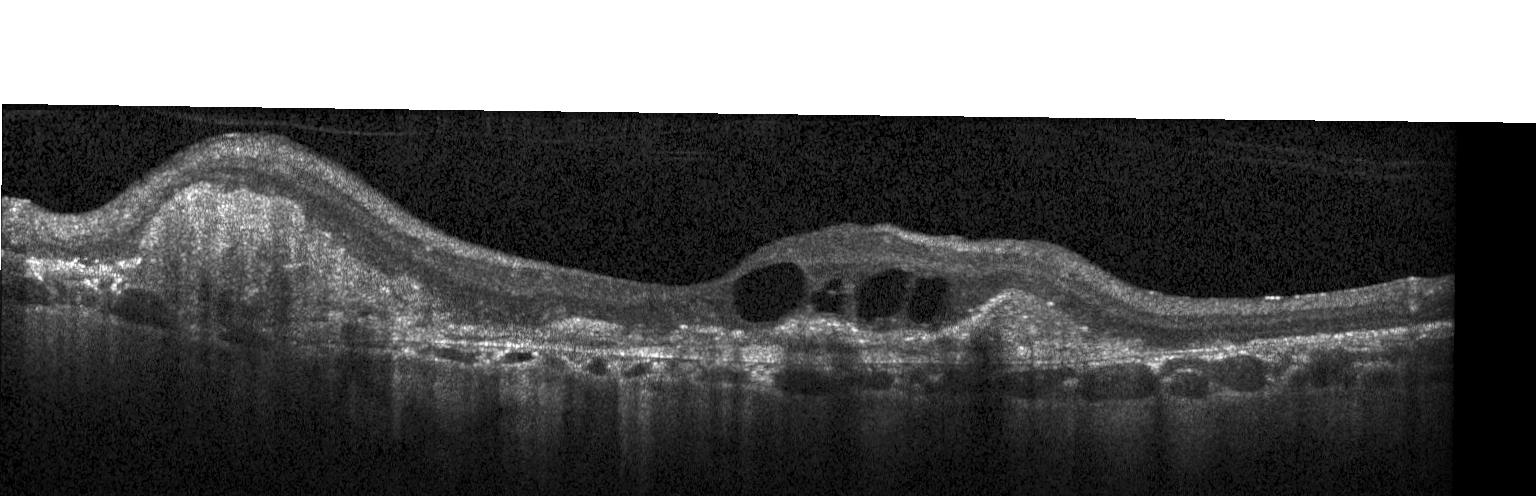

OCT line scan.
Finding: a choroidal neovascular membrane.